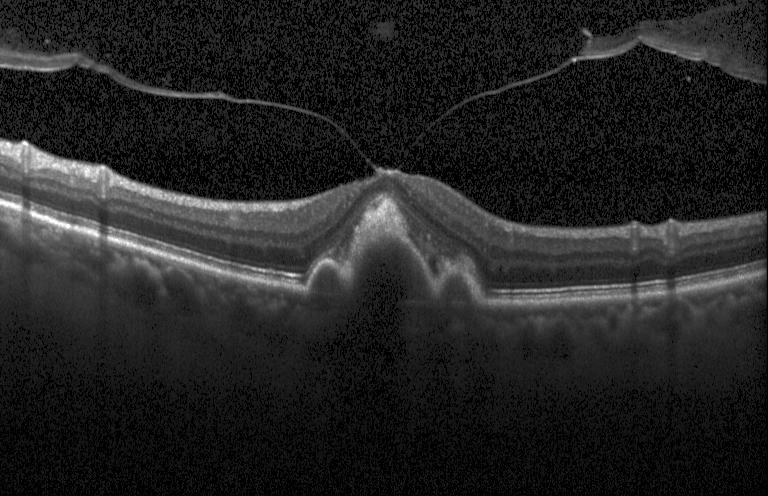

OCT line scan.
The scan shows choroidal neovascularization (CNV).